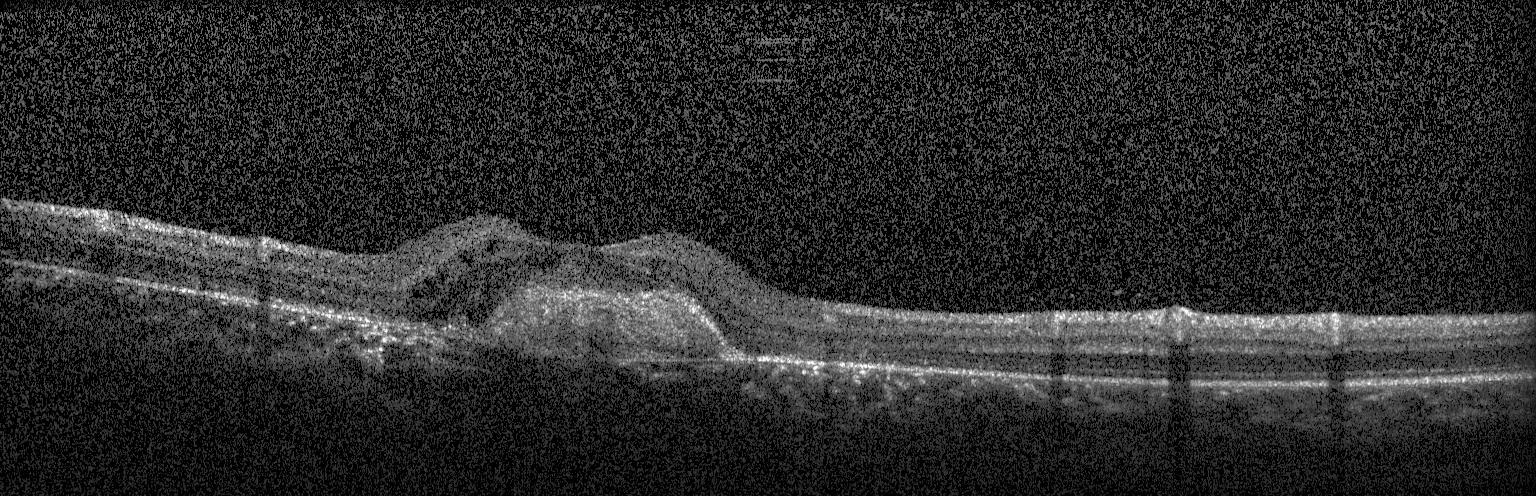 Spectral-domain OCT, through the macula, OCT B-scan. Macular OCT: a choroidal neovascular membrane.